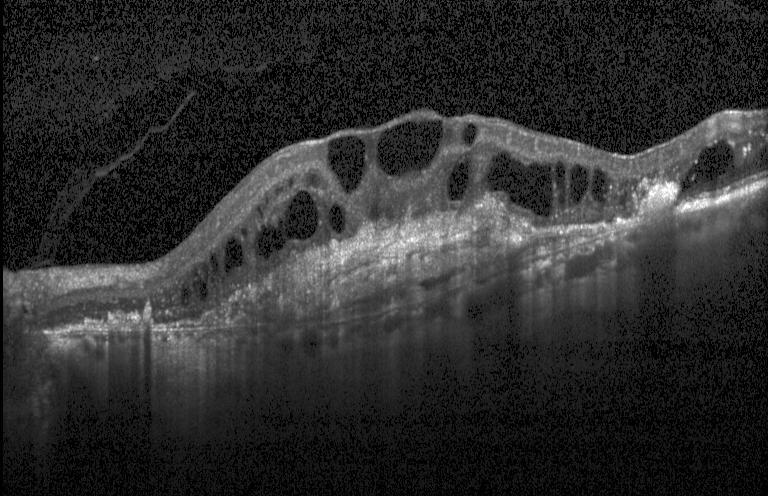

Retinal OCT B-scan. Heidelberg Spectralis OCT system. Through the macula.
Macular OCT: choroidal neovascularization (CNV).